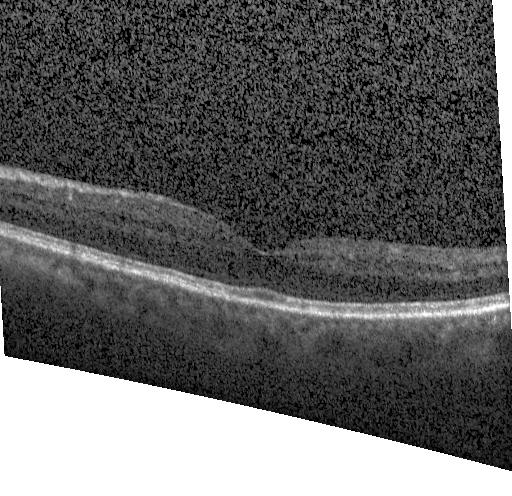
Optical coherence tomography B-scan — Impression: no choroidal neovascularization, diabetic macular edema, or drusen.